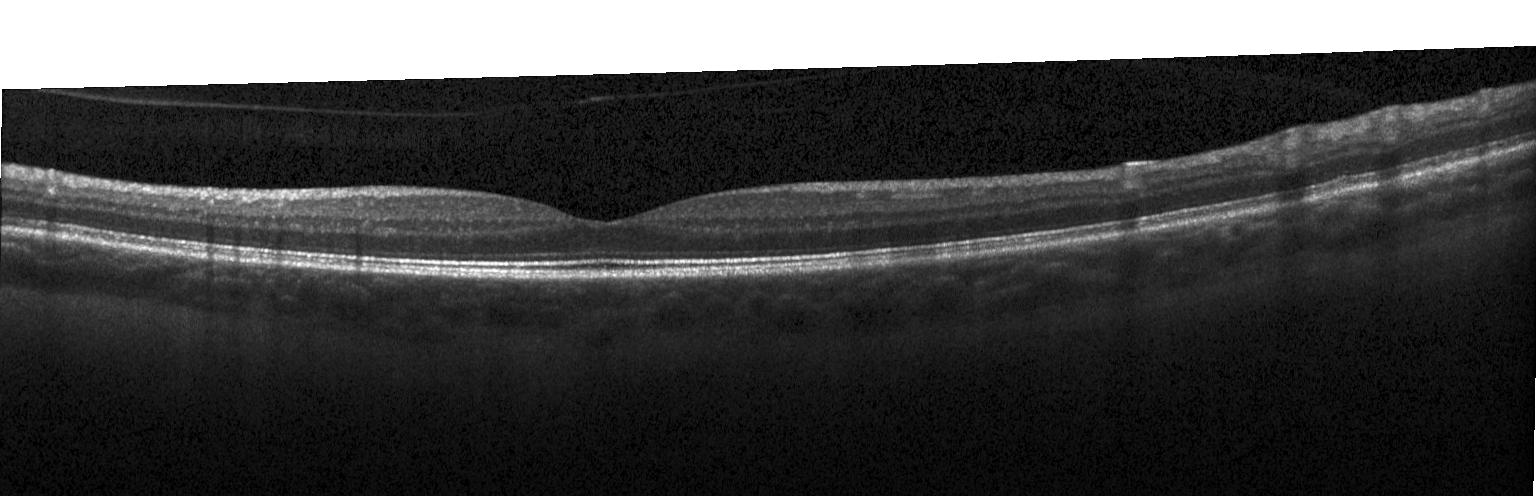
Heidelberg Spectralis OCT system; optical coherence tomography B-scan.
Impression: neither choroidal neovascularization, diabetic macular edema, nor drusen.